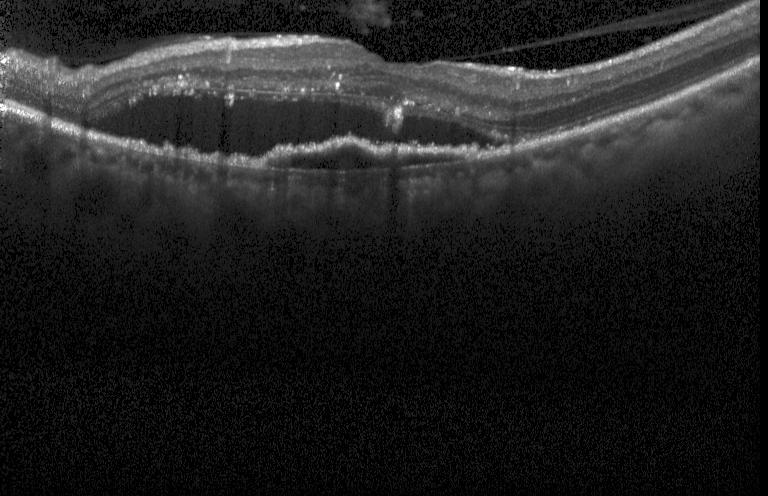
Retinal OCT B-scan.
The scan shows a choroidal neovascular membrane.